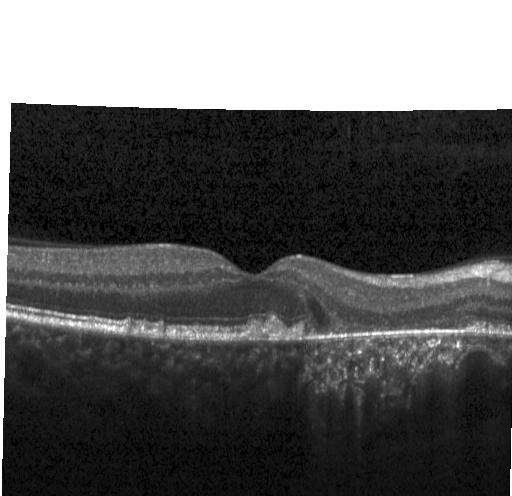
Spectral-domain OCT · horizontal scan through the fovea · optical coherence tomography scan.
Macular OCT: a choroidal neovascular membrane.